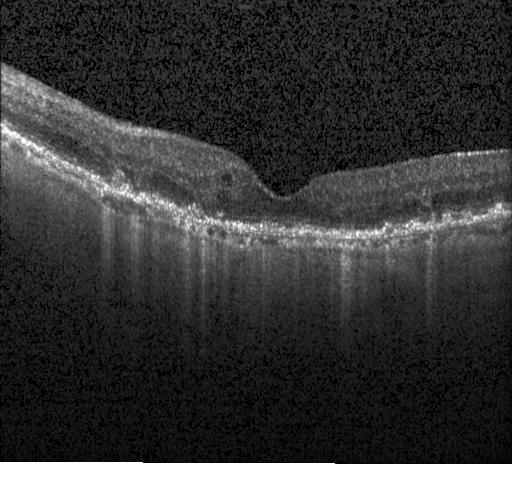 Dx: choroidal neovascularization.